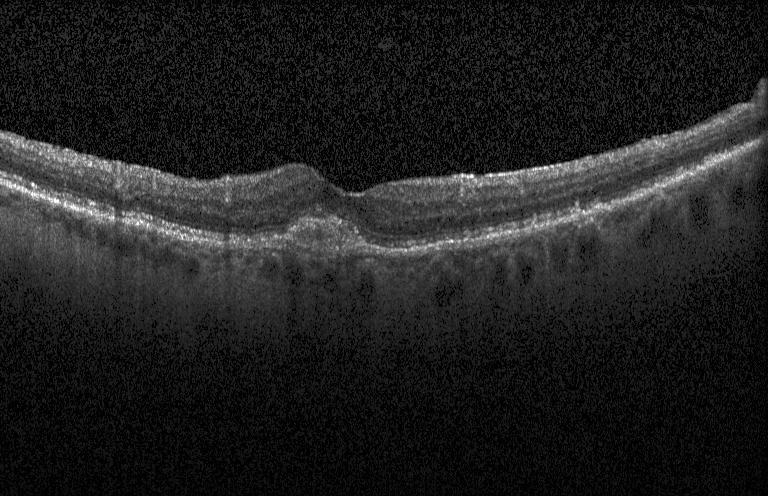
Macular scan; OCT line scan; SD-OCT. Assessment: choroidal neovascularization.